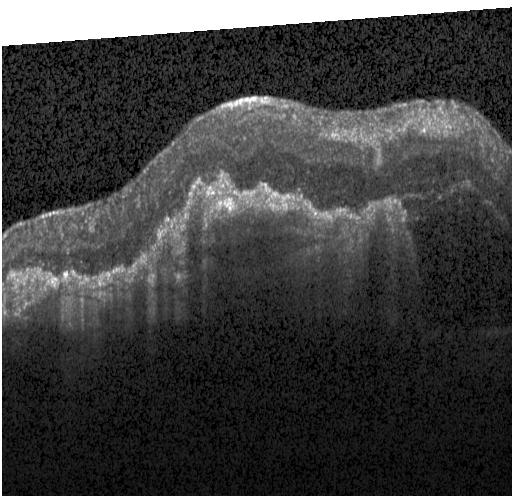
Optical coherence tomography B-scan — Finding: a choroidal neovascular membrane.